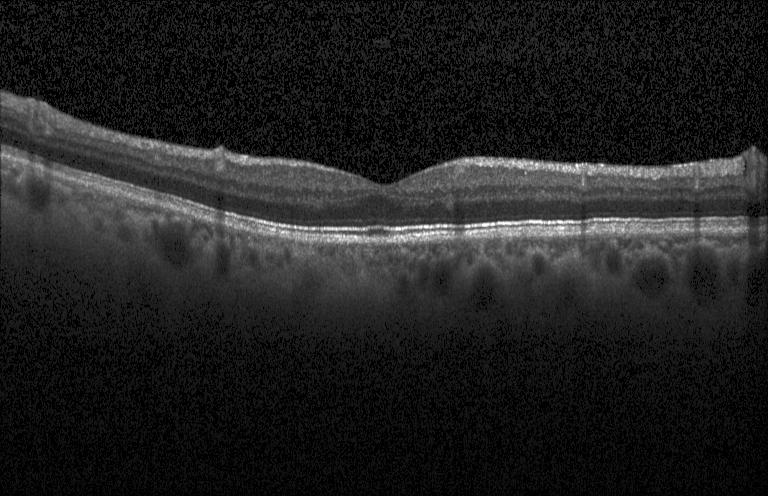
Retinal OCT cross-section; acquired on a Heidelberg Spectralis; spectral-domain optical coherence tomography.
Diagnosis: neither choroidal neovascularization, diabetic macular edema, nor drusen.